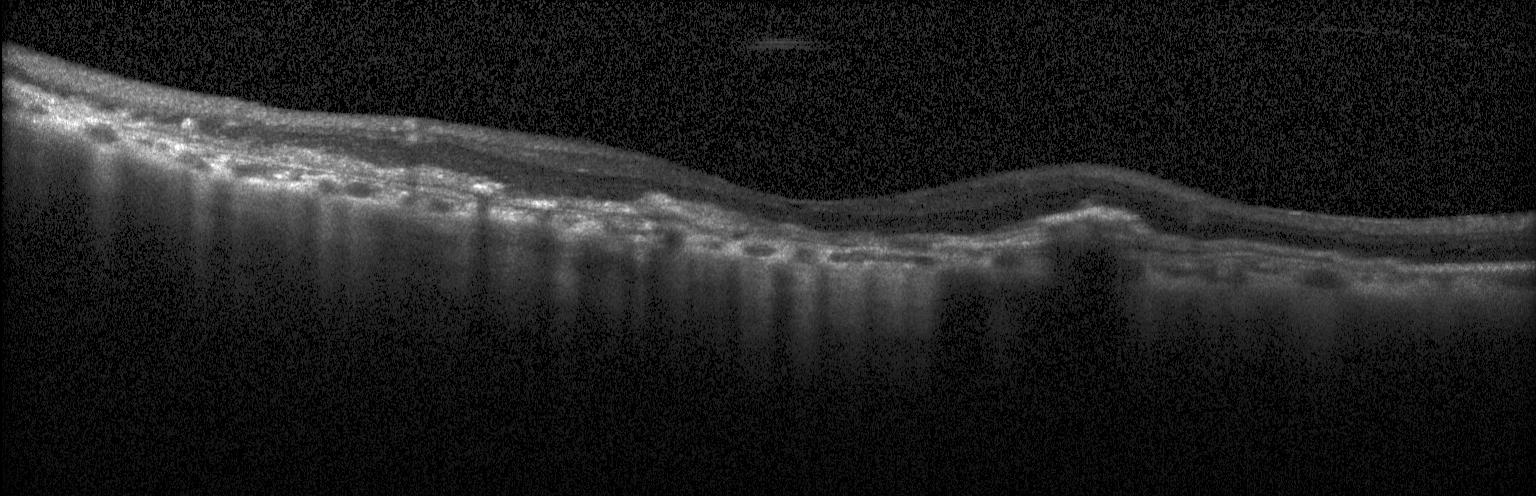
Diagnosis: a choroidal neovascular membrane.